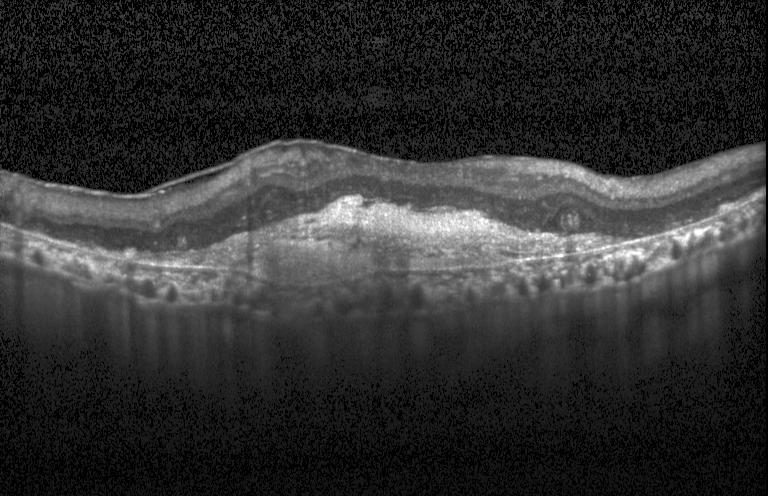

Diagnosis: CNV.